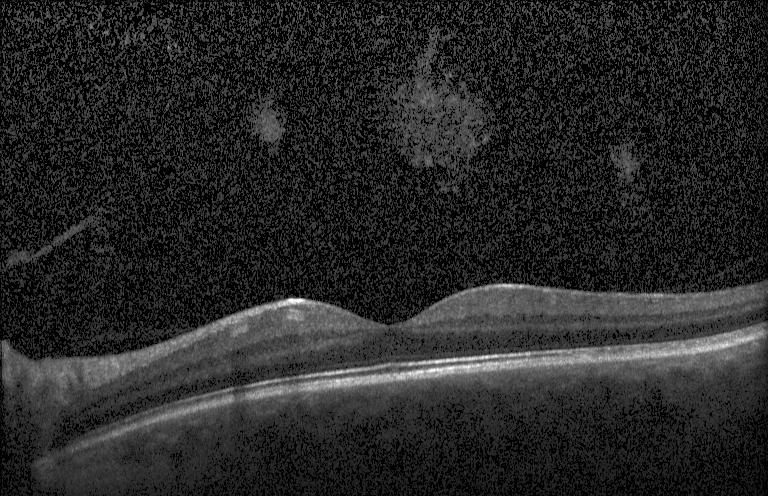 Optical coherence tomography scan. Spectral-domain OCT
Assessment: no CNV, DME, or drusen.